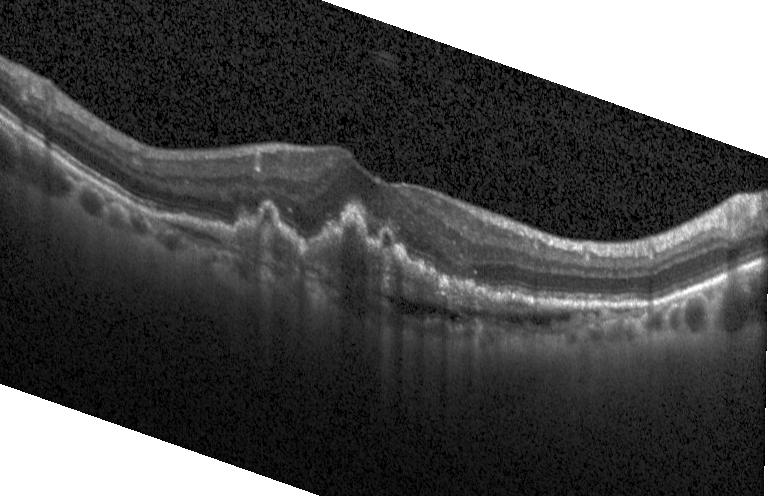 Optical coherence tomography scan · spectral-domain optical coherence tomography · Heidelberg Spectralis OCT system · through the macula. Impression: a choroidal neovascular membrane.